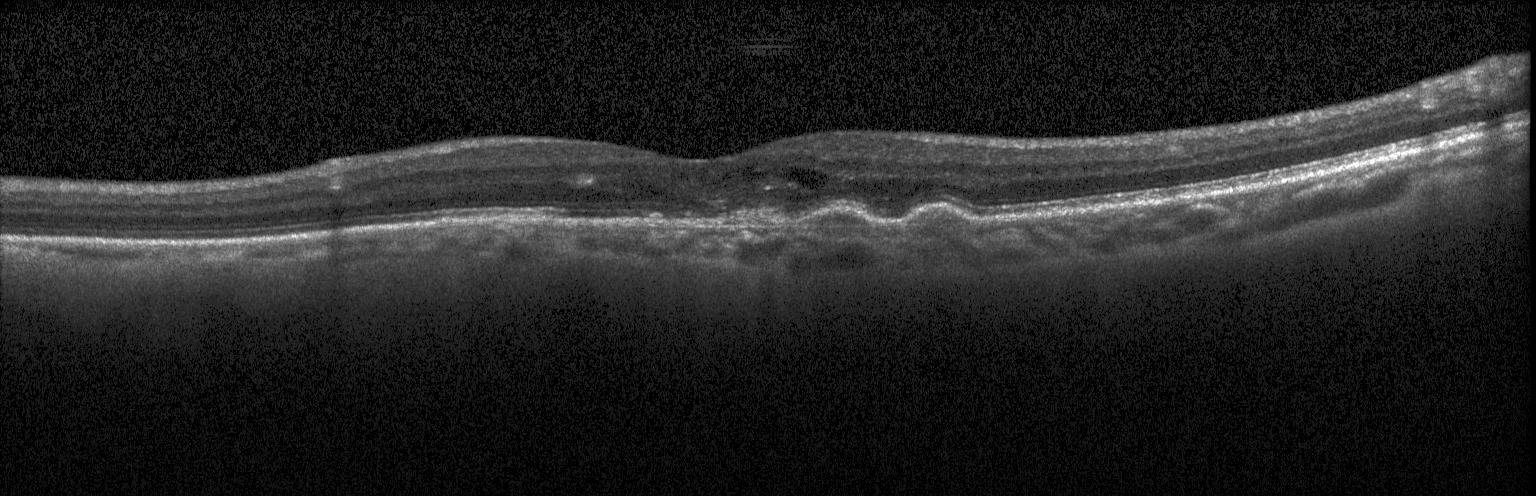
Optical coherence tomography scan.
Impression: CNV.